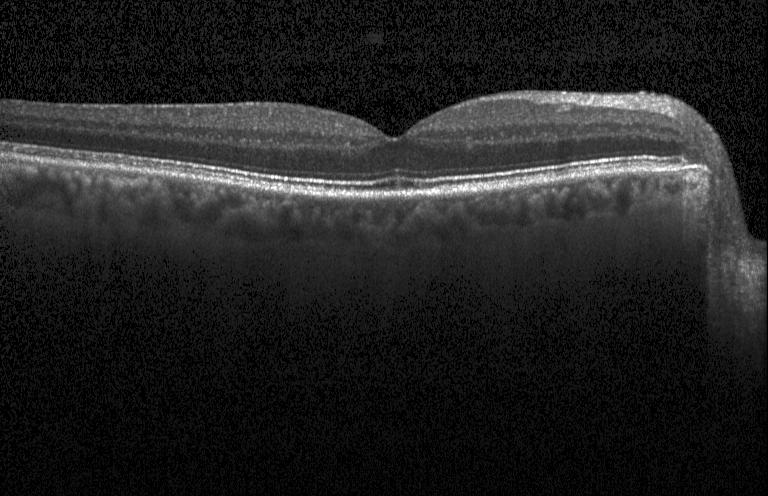
OCT line scan.
Impression: no evidence of choroidal neovascularization, diabetic macular edema, or drusen.